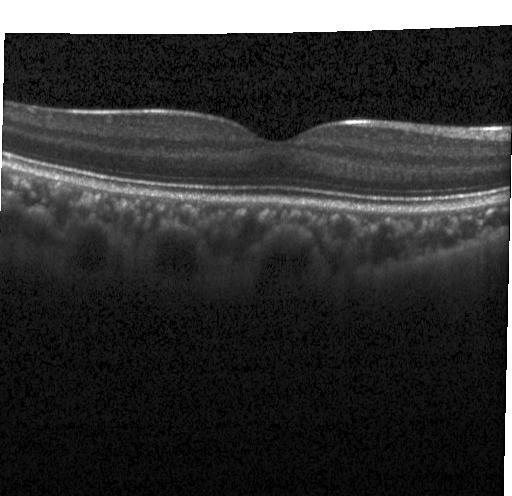

Assessment: no evidence of choroidal neovascularization, diabetic macular edema, or drusen.